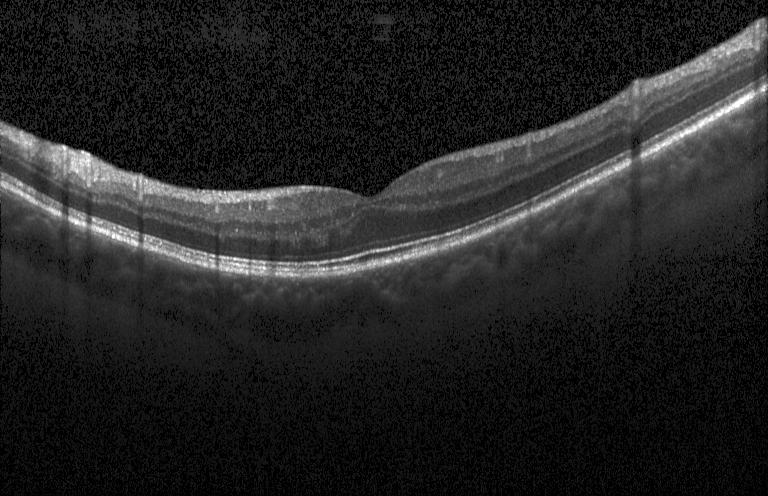
Spectral-domain optical coherence tomography, retinal OCT B-scan.
Impression: no choroidal neovascularization, no diabetic macular edema, and no drusen.